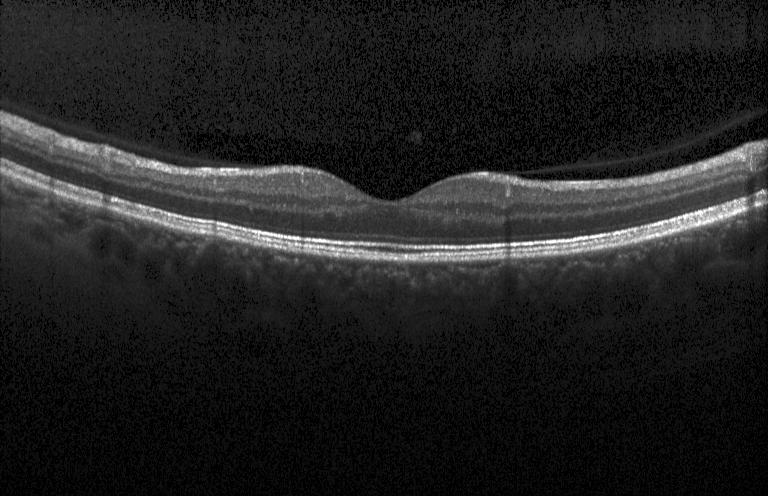

Spectral-domain OCT, Heidelberg Spectralis OCT system, fovea-centered, optical coherence tomography B-scan
Finding: no CNV, no DME, and no drusen.